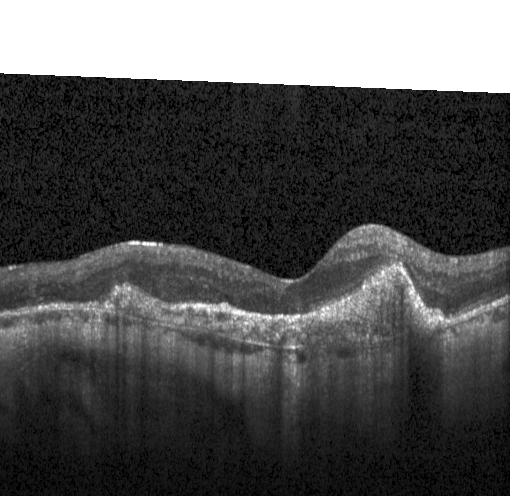 Optical coherence tomography B-scan · SD-OCT. Impression: a choroidal neovascular membrane.